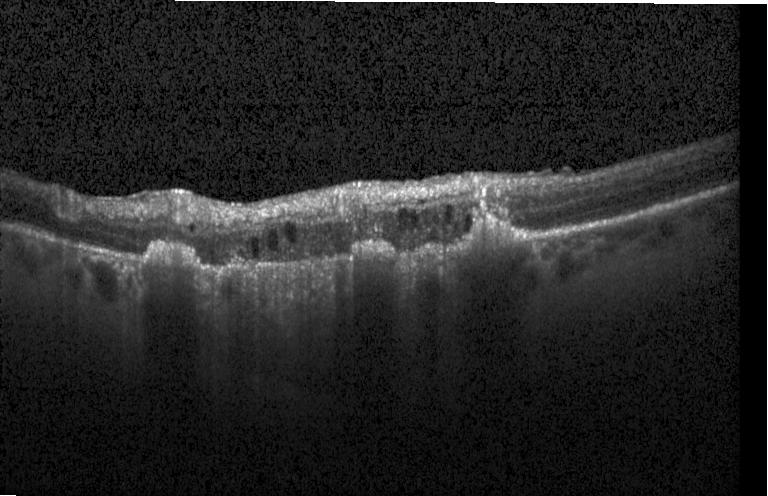
Finding: choroidal neovascularization.